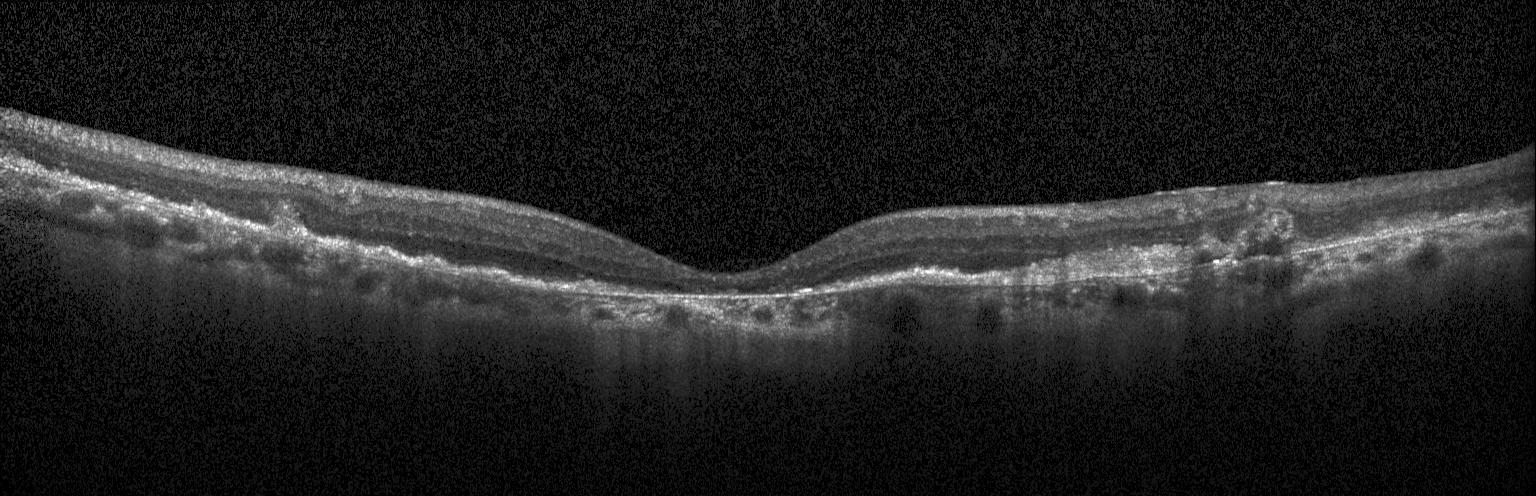
OCT B-scan. Diagnosis: a choroidal neovascular membrane.